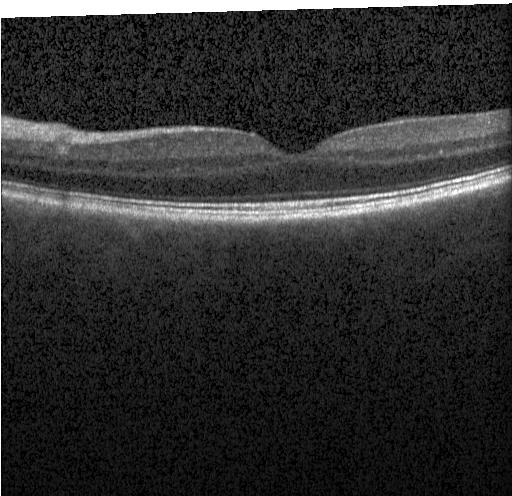
Retinal OCT B-scan; fovea-centered
Finding: no evidence of CNV, DME, or drusen.